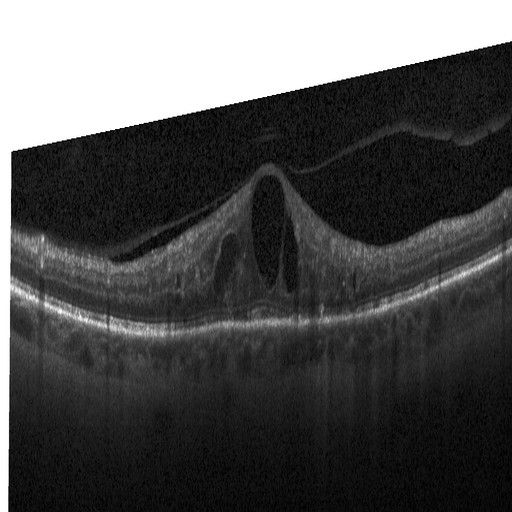 Spectral-domain optical coherence tomography · retinal OCT B-scan · instrument: Heidelberg Spectralis · centered on the fovea. Dx: diabetic macular edema.